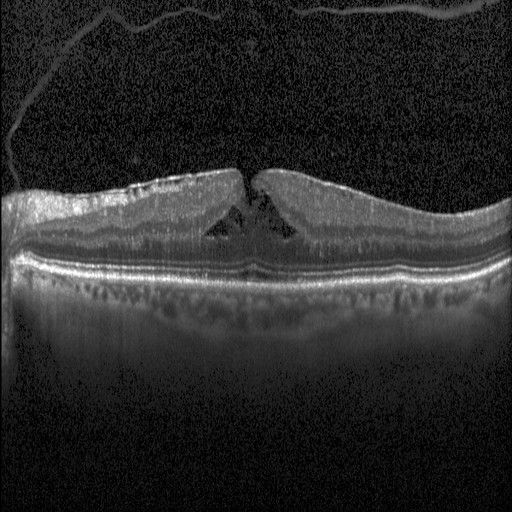

OCT finding: DME.